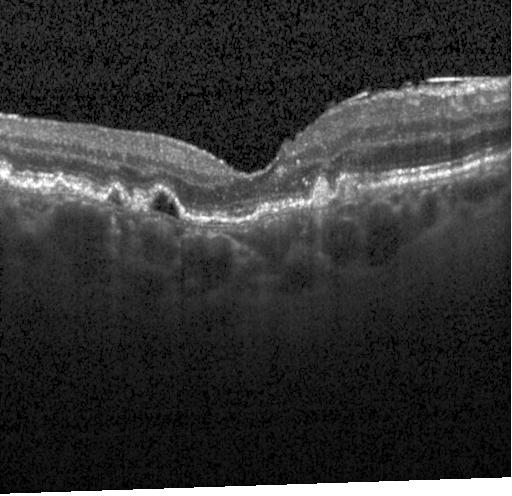 OCT finding: choroidal neovascularization.